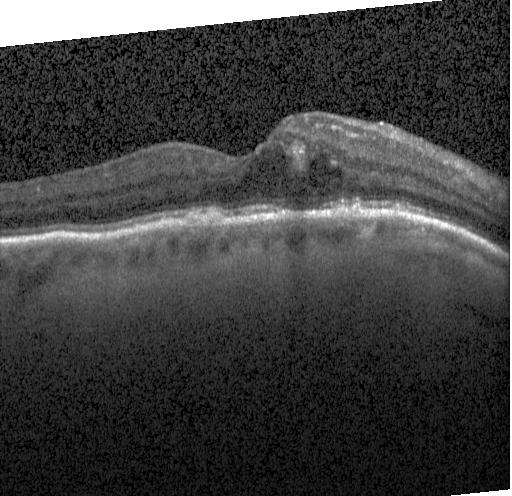 Acquired on a Heidelberg Spectralis. Horizontal scan through the fovea. Spectral-domain optical coherence tomography. Optical coherence tomography scan. The scan shows CNV.